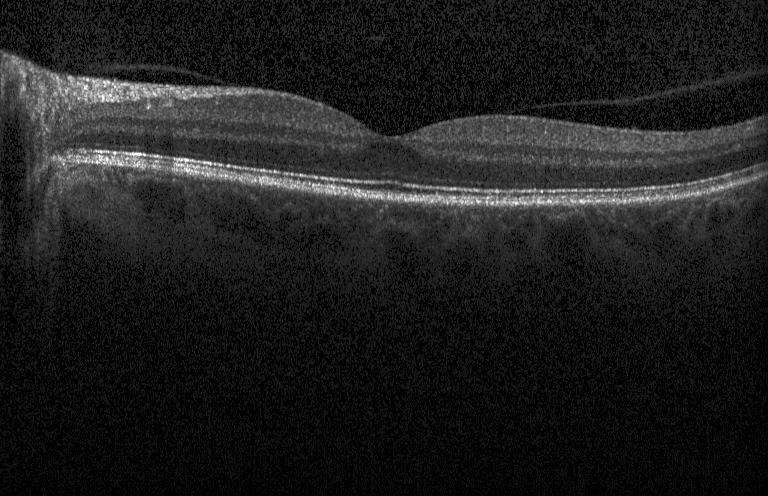
No evidence of CNV, DME, or drusen.